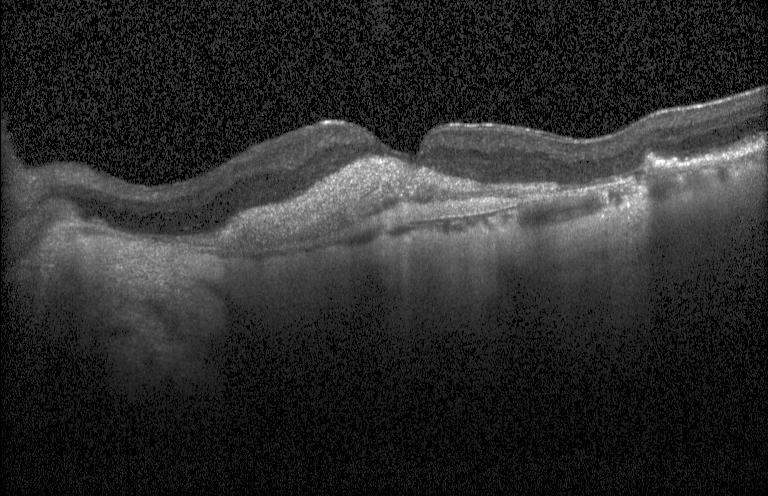

Retinal OCT B-scan. Impression: a choroidal neovascular membrane.